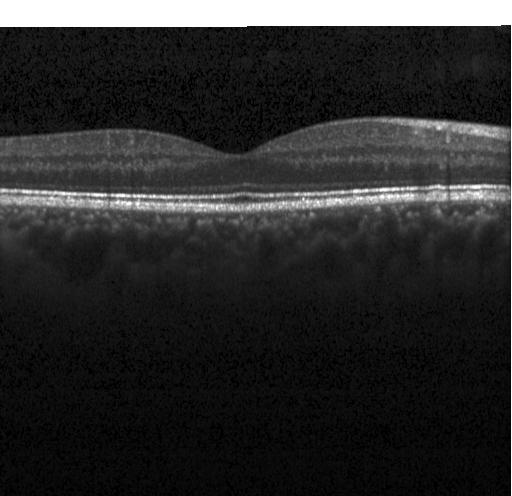
Heidelberg Spectralis OCT system · spectral-domain optical coherence tomography · optical coherence tomography scan
Impression: neither choroidal neovascularization, diabetic macular edema, nor drusen.